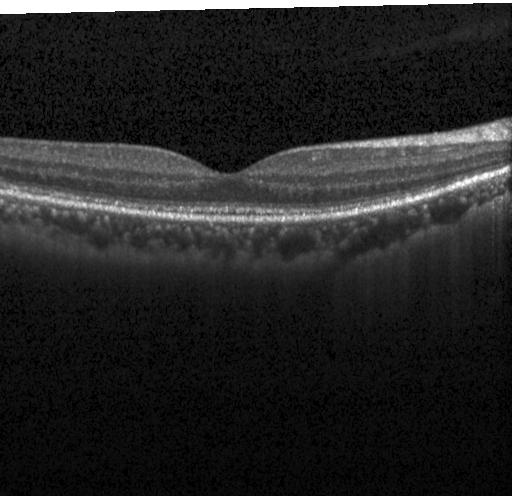
Retinal OCT cross-section.
Diagnosis: no choroidal neovascularization, no diabetic macular edema, and no drusen.